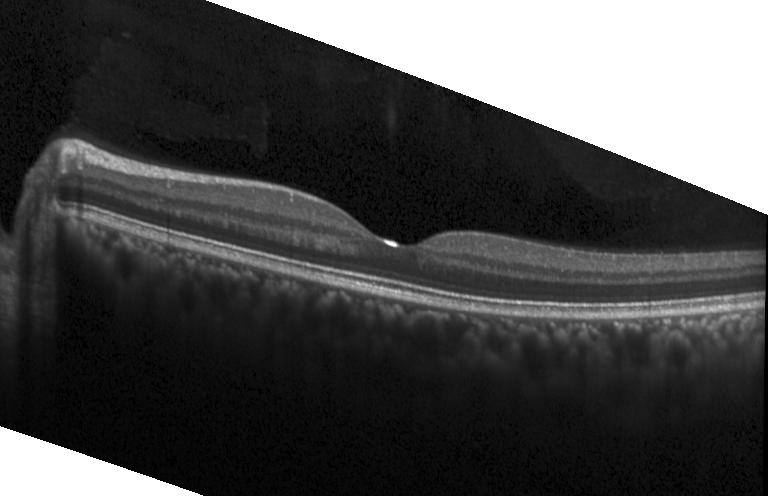
Spectral-domain optical coherence tomography · retinal OCT B-scan. OCT finding: no evidence of choroidal neovascularization, diabetic macular edema, or drusen.